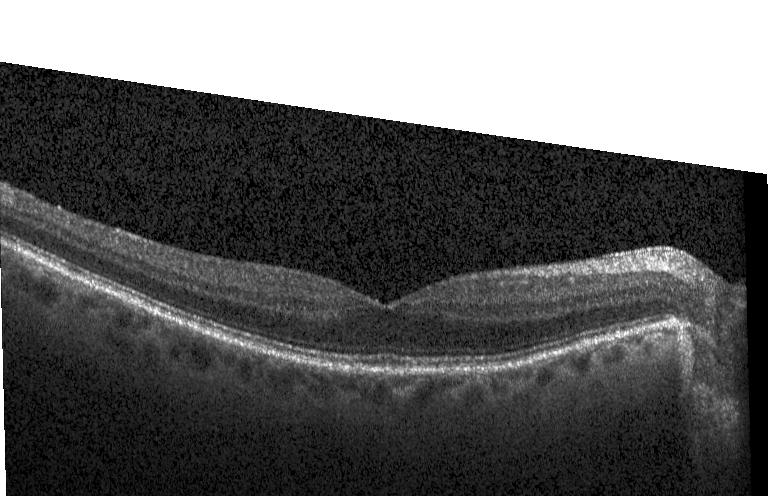
SD-OCT; Heidelberg Spectralis; OCT B-scan — Finding: no choroidal neovascularization, no diabetic macular edema, and no drusen.